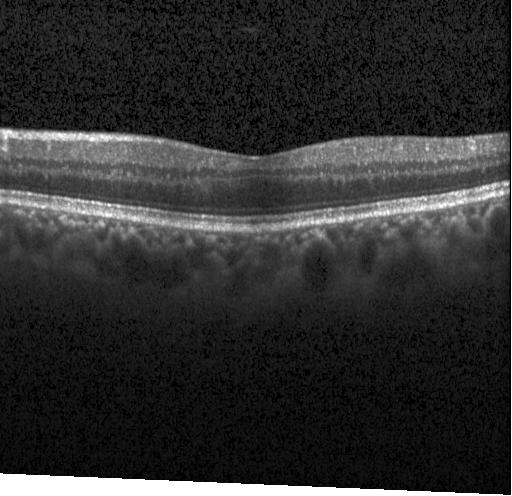

Instrument: Heidelberg Spectralis, horizontal scan through the fovea, retinal OCT B-scan.
Dx: no evidence of choroidal neovascularization, diabetic macular edema, or drusen.